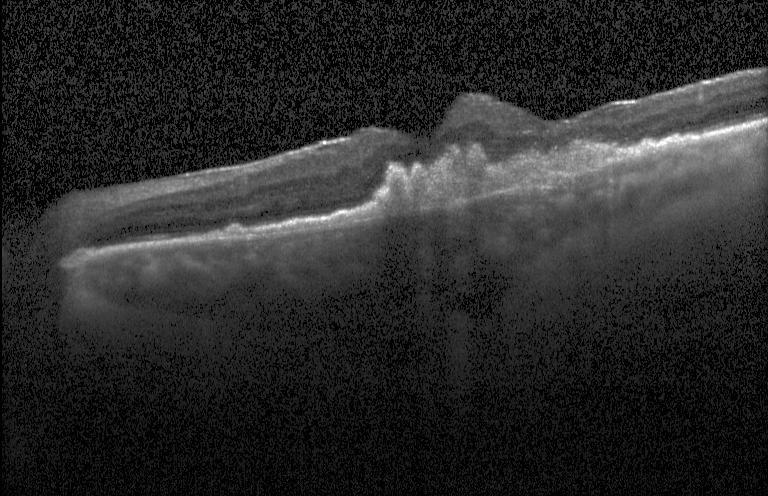 Spectral-domain optical coherence tomography · OCT line scan — Dx: choroidal neovascularization.